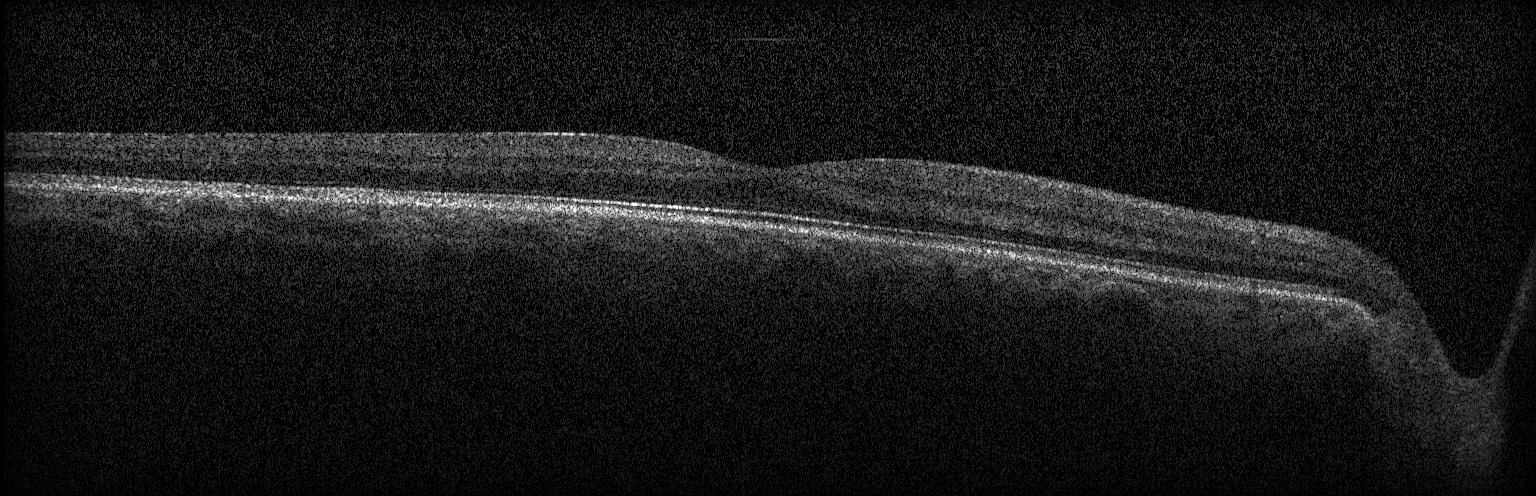 Spectral-domain OCT · Heidelberg Spectralis · optical coherence tomography scan
Macular OCT: no CNV, DME, or drusen.